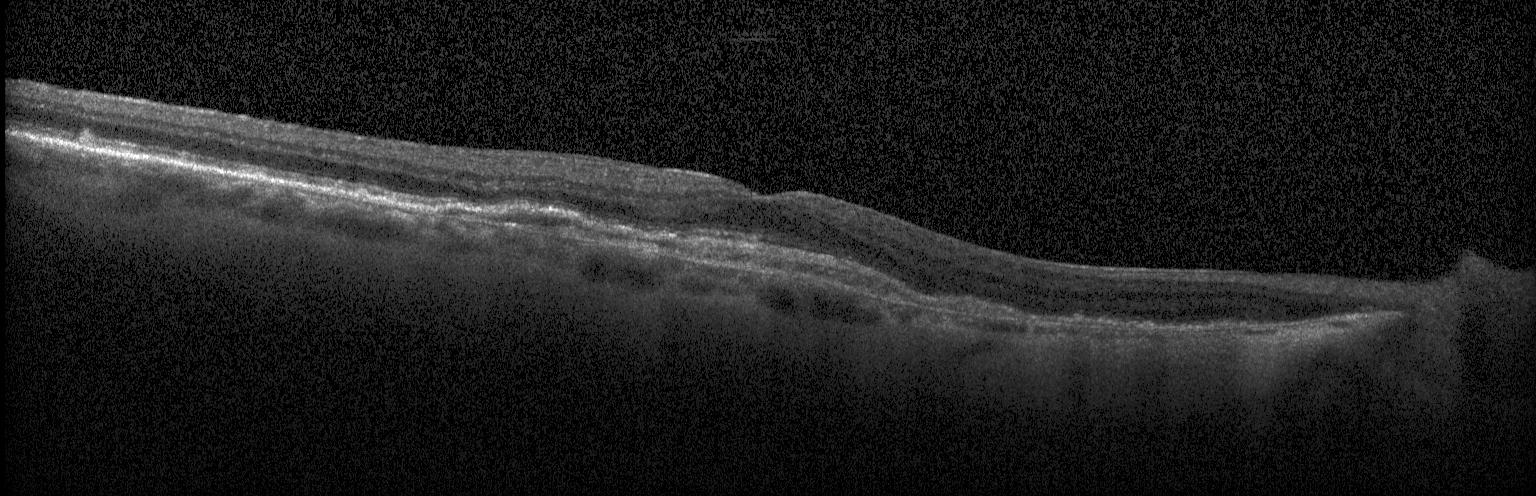
Diagnosis: a choroidal neovascular membrane.